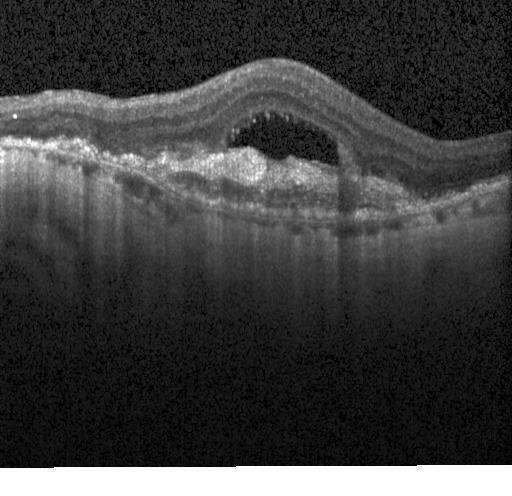 SD-OCT · instrument: Heidelberg Spectralis · macular scan · retinal OCT B-scan.
Impression: a choroidal neovascular membrane.